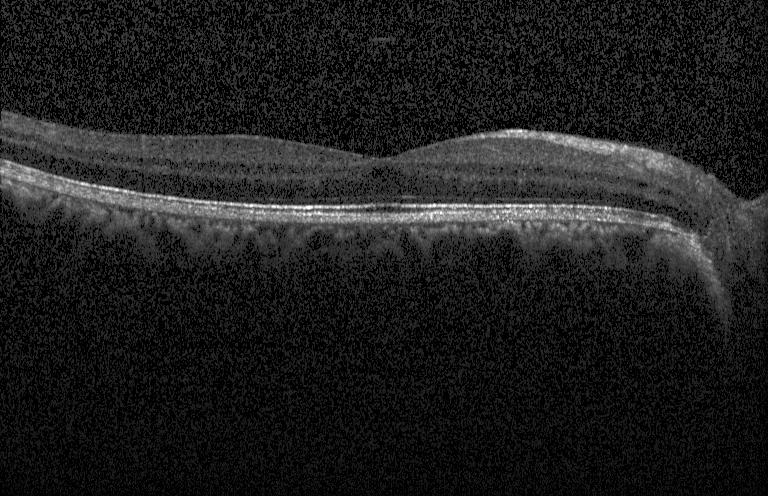
Assessment: no CNV, no DME, and no drusen.